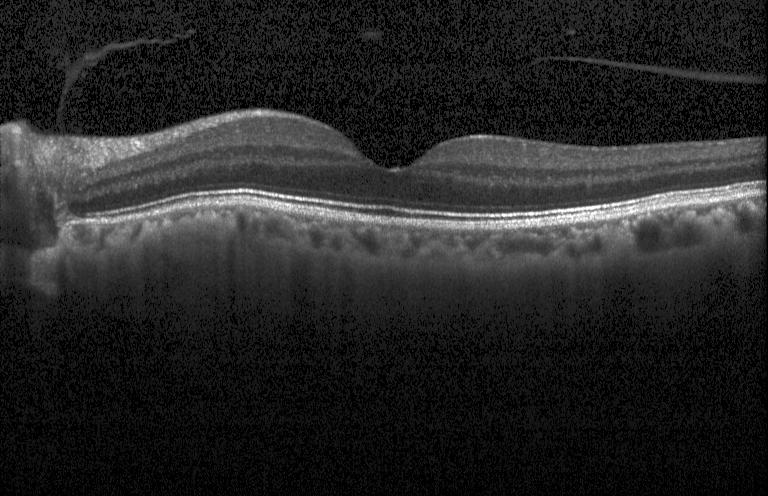 Impression: neither CNV, DME, nor drusen.